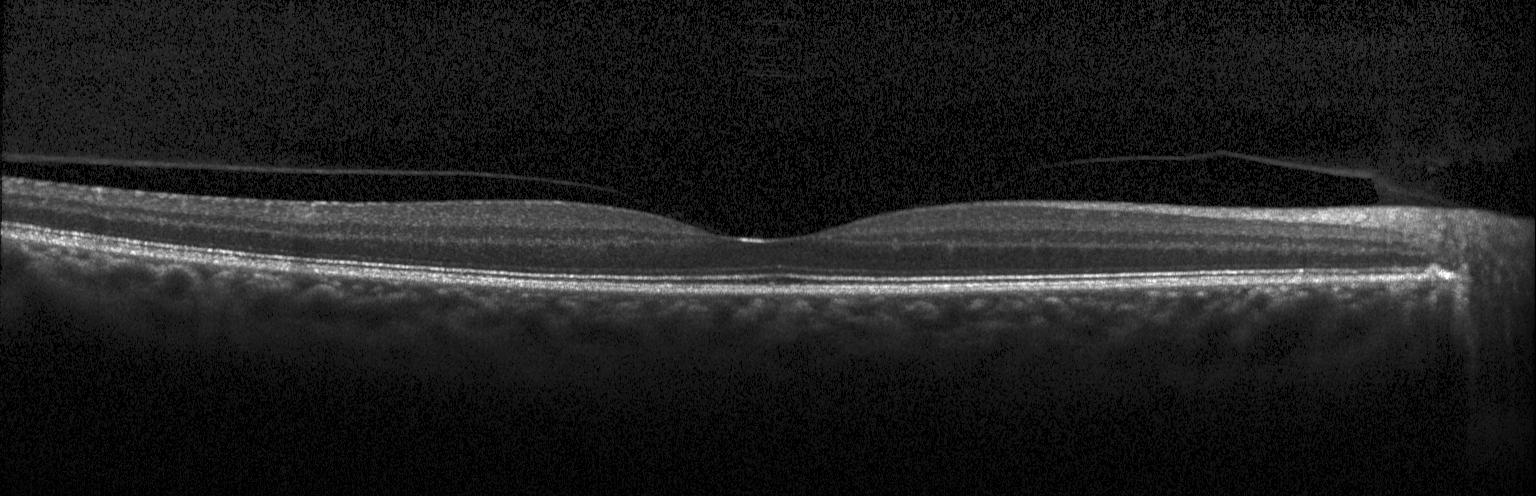

This B-scan demonstrates no choroidal neovascularization, no diabetic macular edema, and no drusen.